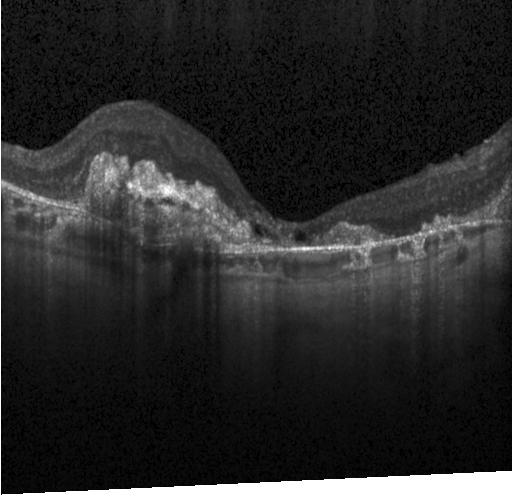 Spectral-domain OCT B-scan: choroidal neovascularization.